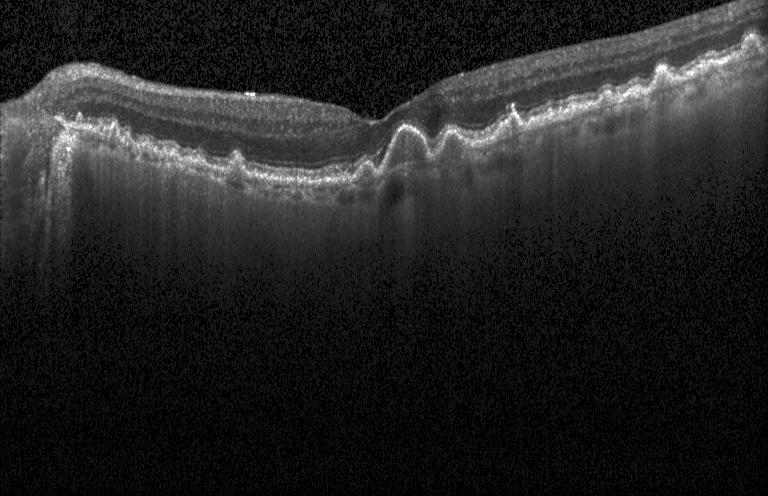

Spectral-domain OCT B-scan: multiple drusen.